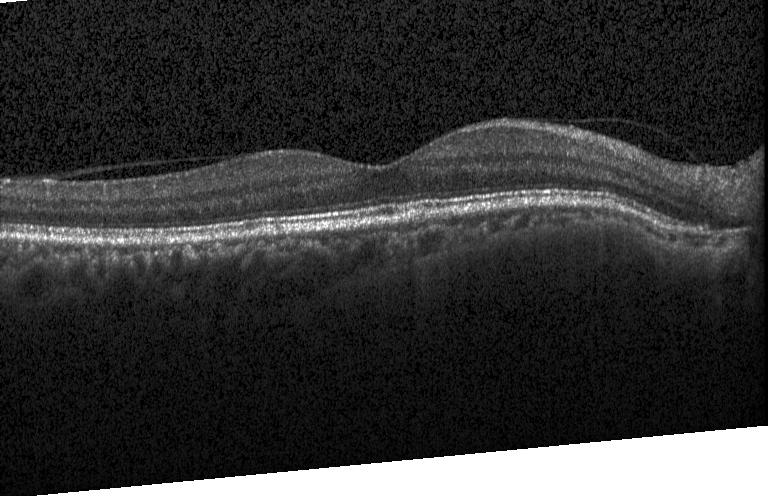

Diagnosis: no CNV, no DME, and no drusen.